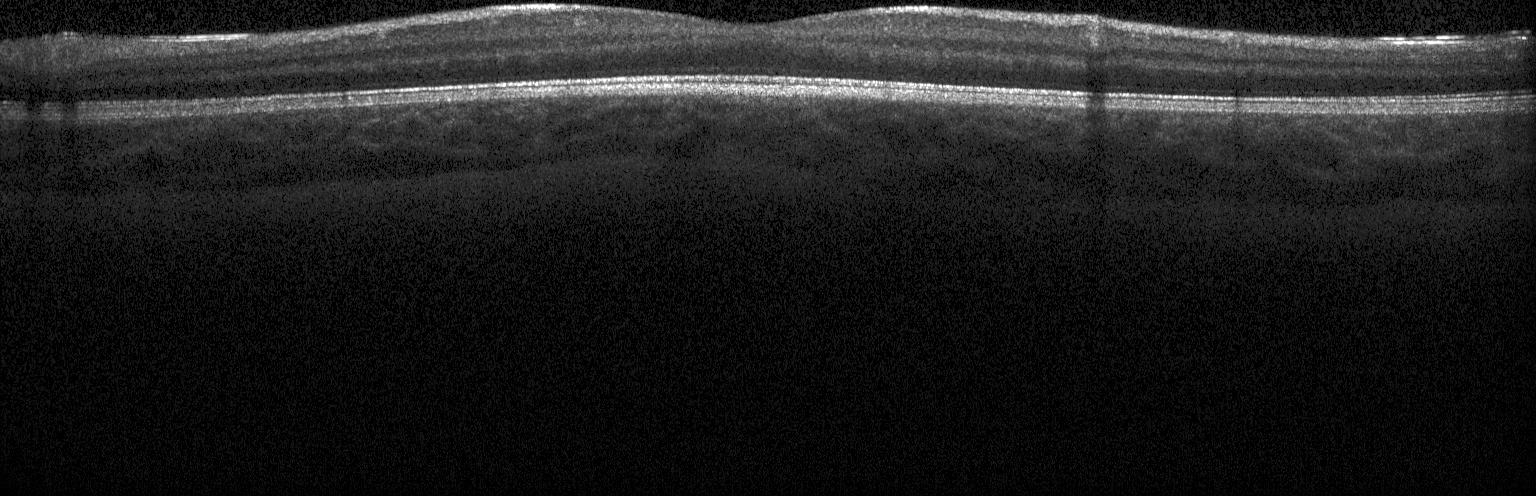 Finding: no choroidal neovascularization, diabetic macular edema, or drusen.